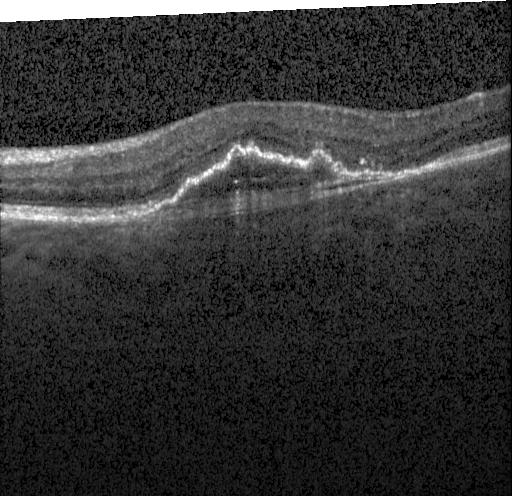 Spectral-domain OCT; optical coherence tomography B-scan.
Impression: CNV.